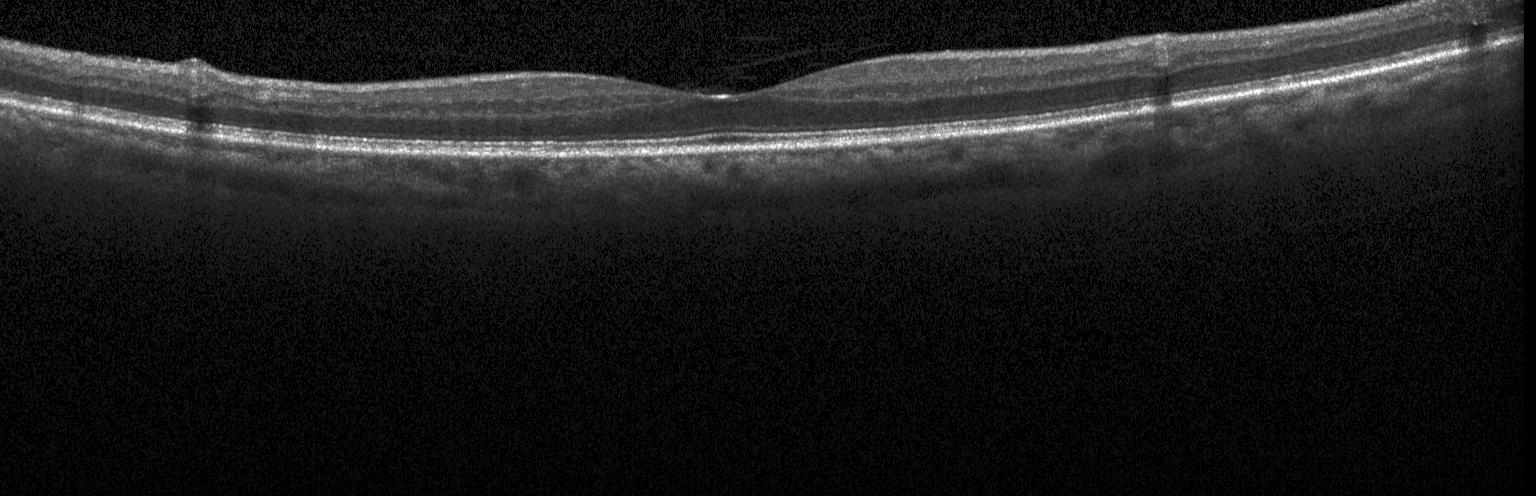 OCT line scan — Impression: no evidence of choroidal neovascularization, diabetic macular edema, or drusen.